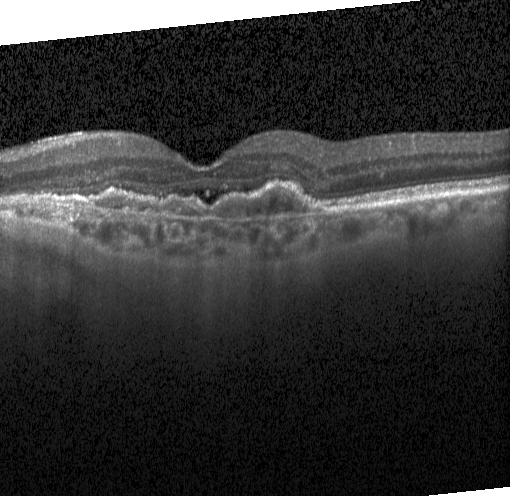
Spectral-domain OCT · OCT line scan. This B-scan demonstrates a choroidal neovascular membrane.